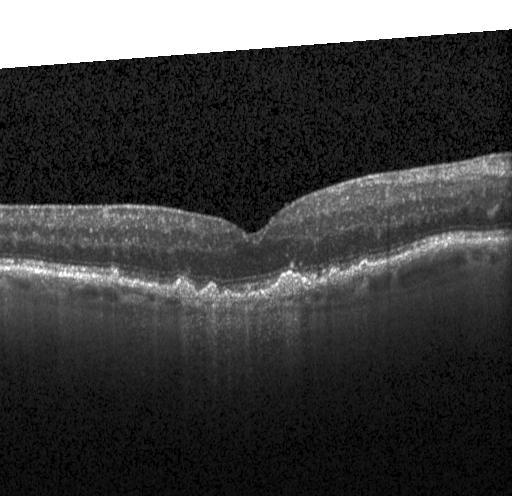 OCT B-scan showing a choroidal neovascular membrane.